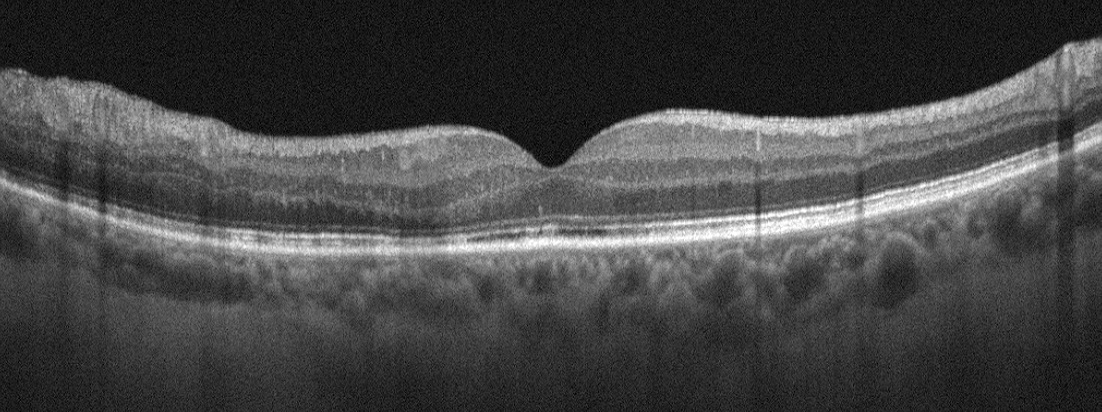

Optovue Avanti RTVue XR. Retinal OCT B-scan. Diagnosis: diabetic macular edema.